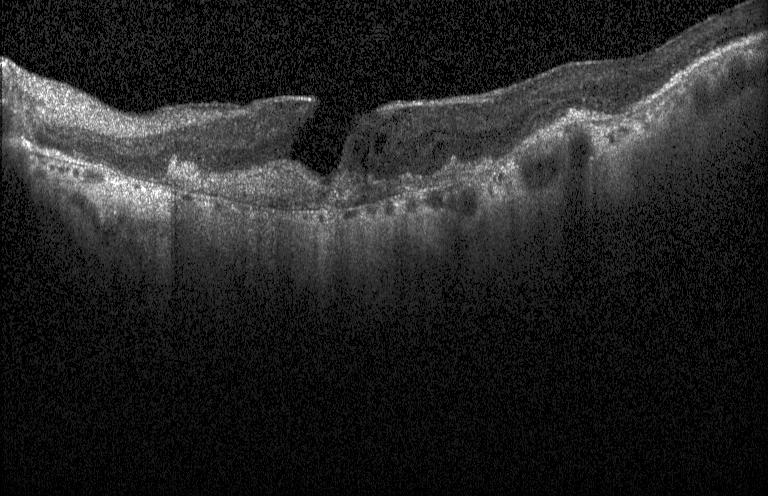

OCT B-scan, Heidelberg Spectralis OCT system — Macular OCT: choroidal neovascularization.